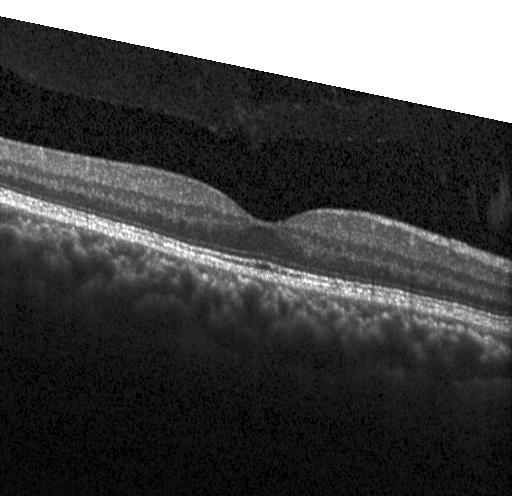
Assessment: no choroidal neovascularization, diabetic macular edema, or drusen.